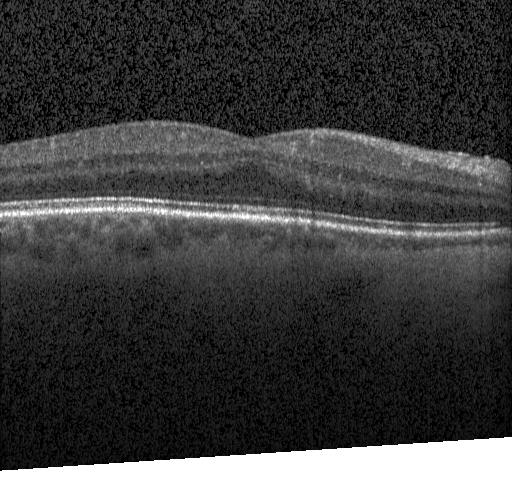 Finding: no evidence of choroidal neovascularization, diabetic macular edema, or drusen.